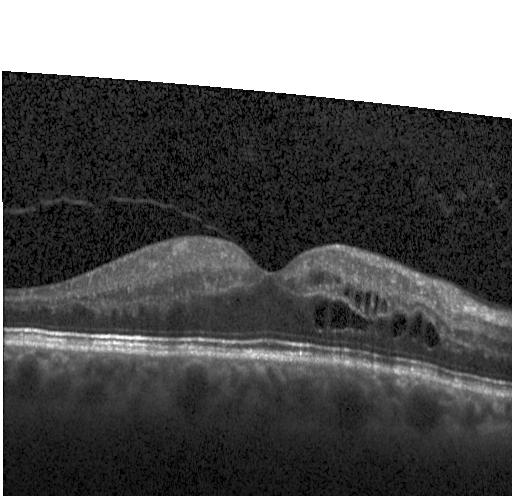

OCT line scan.
Diabetic macular edema (DME).